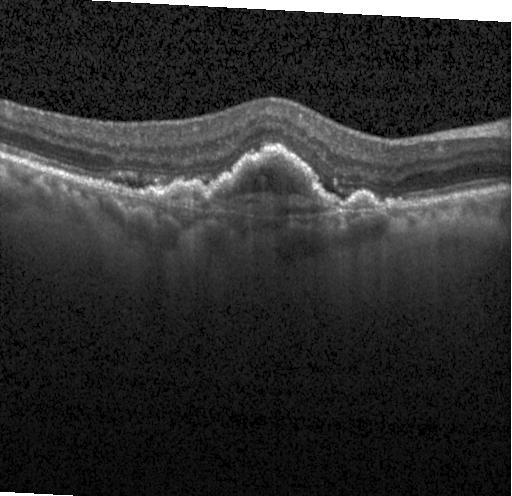
OCT line scan · spectral-domain optical coherence tomography · Heidelberg Spectralis OCT system — Impression: a choroidal neovascular membrane.